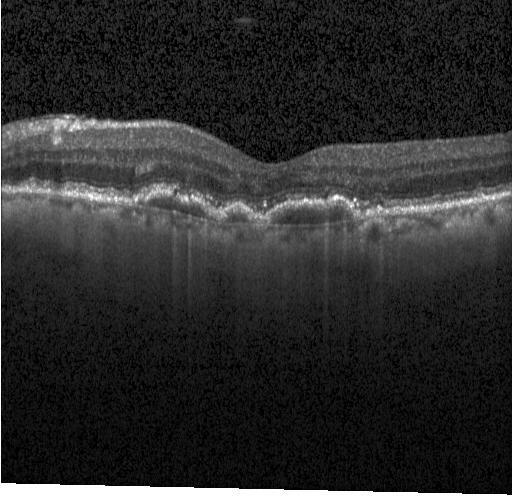
Finding: choroidal neovascularization (CNV).